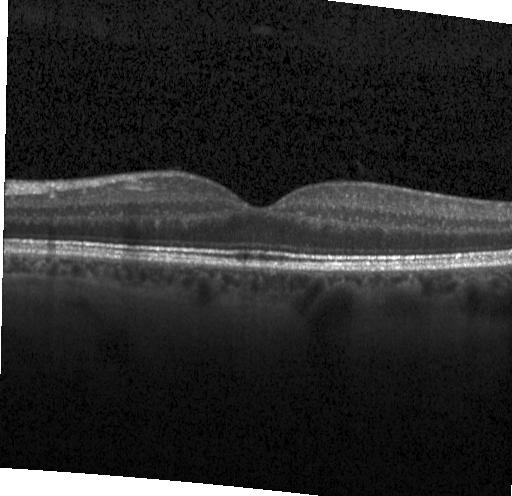 OCT B-scan showing no choroidal neovascularization, no diabetic macular edema, and no drusen.